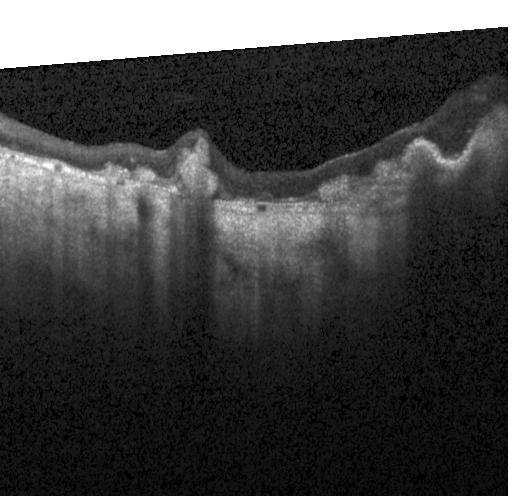

Heidelberg Spectralis · spectral-domain optical coherence tomography · optical coherence tomography scan. This B-scan demonstrates a choroidal neovascular membrane.